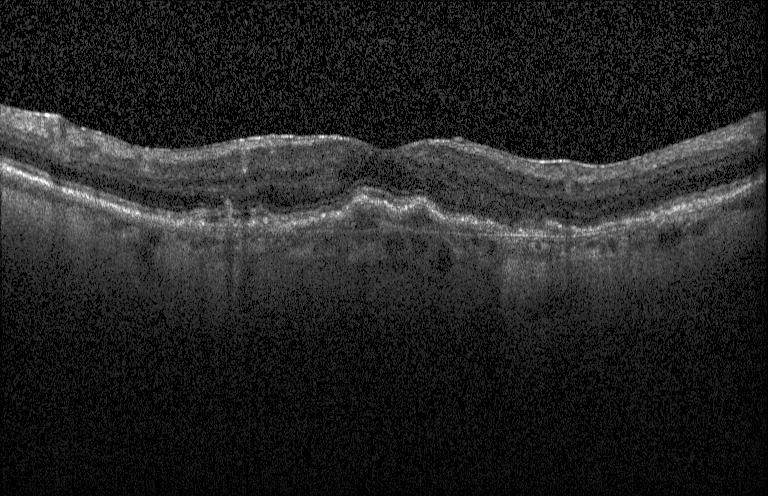 Optical coherence tomography scan.
Impression: a choroidal neovascular membrane.